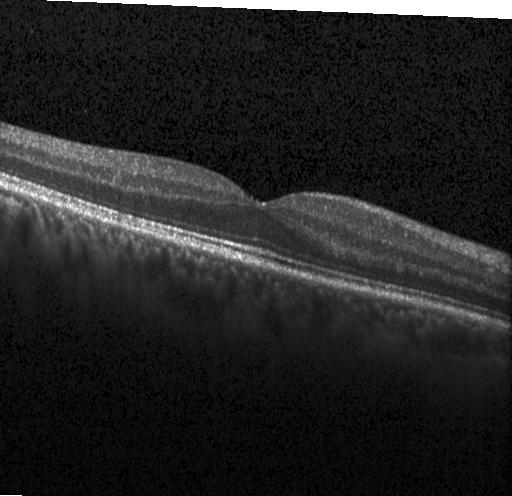

Impression: neither choroidal neovascularization, diabetic macular edema, nor drusen.